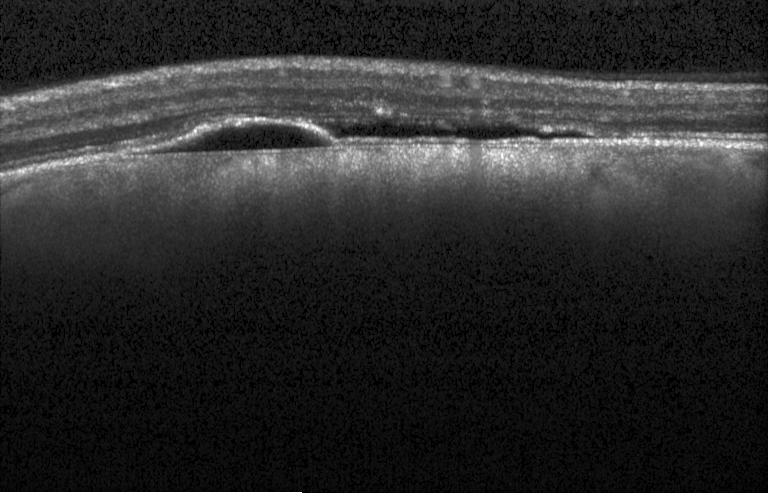
Retinal OCT cross-section.
Dx: a choroidal neovascular membrane.